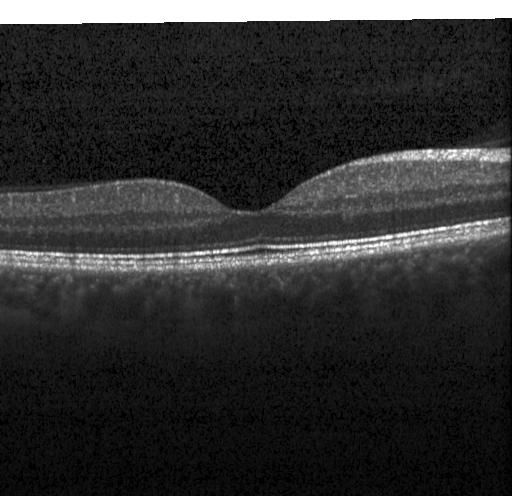
OCT B-scan
Impression: neither choroidal neovascularization, diabetic macular edema, nor drusen.